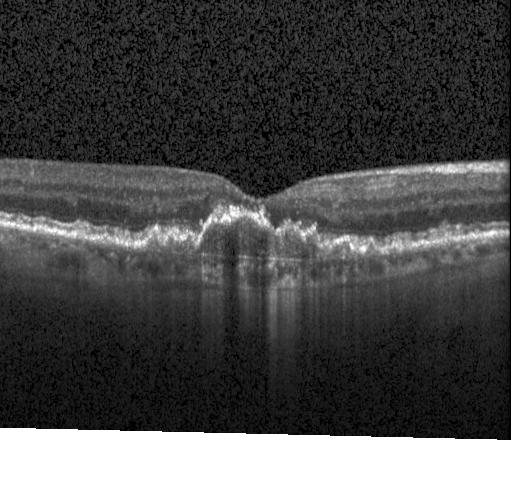
Spectral-domain OCT B-scan: CNV.